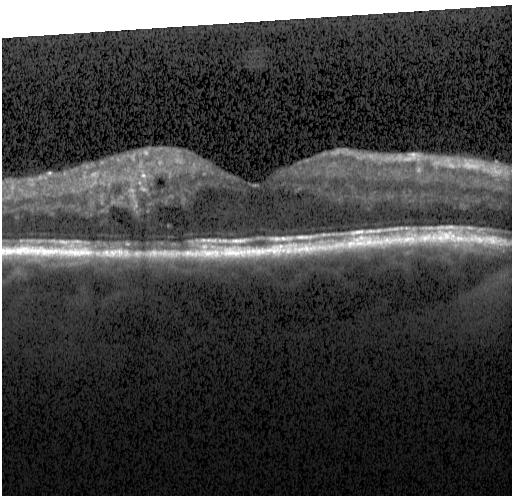

SD-OCT; through the macula; retinal OCT B-scan; instrument: Heidelberg Spectralis — Diagnosis: diabetic macular edema (DME).